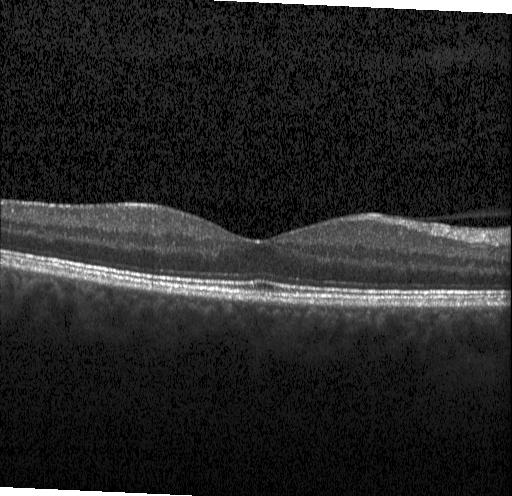 Optical coherence tomography B-scan, SD-OCT, instrument: Heidelberg Spectralis — Macular OCT: no evidence of CNV, DME, or drusen.